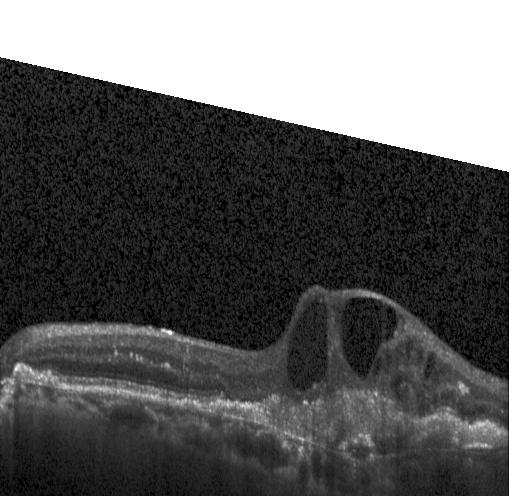

OCT B-scan, SD-OCT, through the macula, instrument: Heidelberg Spectralis
OCT finding: a choroidal neovascular membrane.